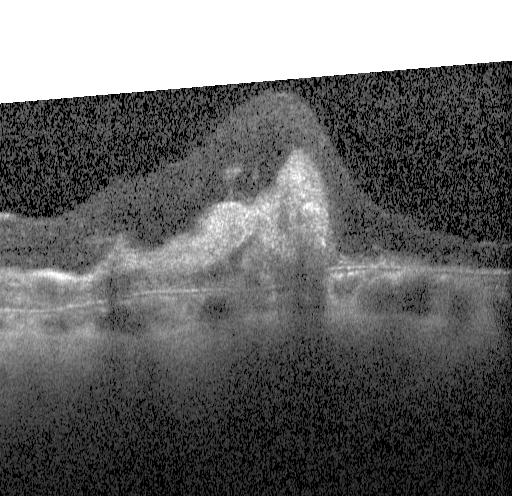 Finding: choroidal neovascularization.